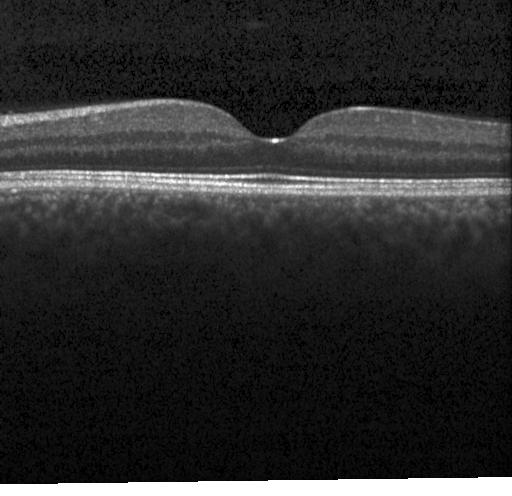 Retinal OCT B-scan, SD-OCT, through the macula.
Diagnosis: neither choroidal neovascularization, diabetic macular edema, nor drusen.